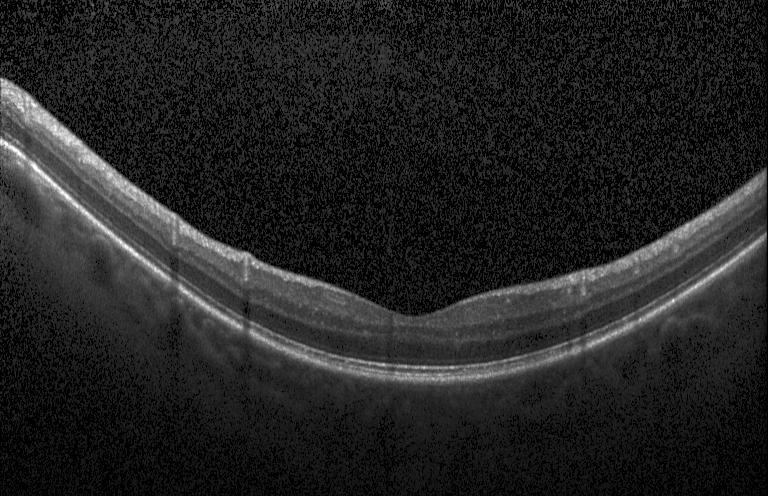

Dx: neither choroidal neovascularization, diabetic macular edema, nor drusen.